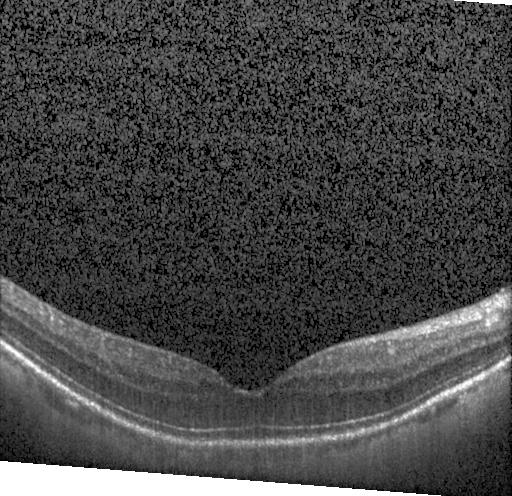

The scan shows neither choroidal neovascularization, diabetic macular edema, nor drusen.